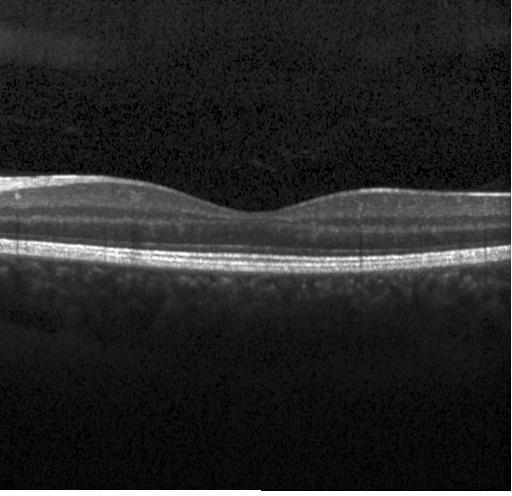 OCT line scan.
Dx: no evidence of CNV, DME, or drusen.